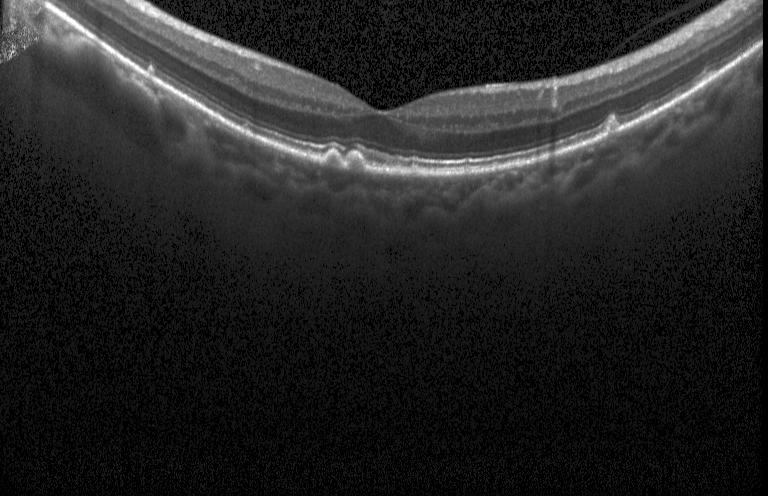

OCT line scan; through the macula.
Macular OCT: drusen.